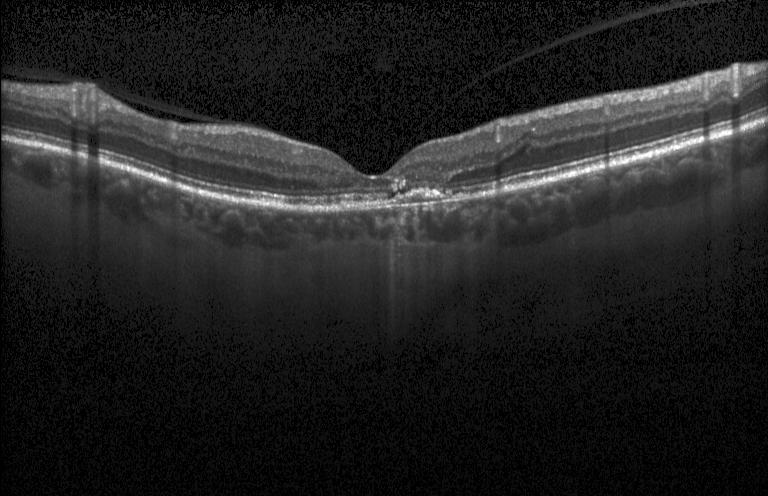

Centered on the fovea. OCT line scan. Spectral-domain OCT — The scan shows choroidal neovascularization (CNV).